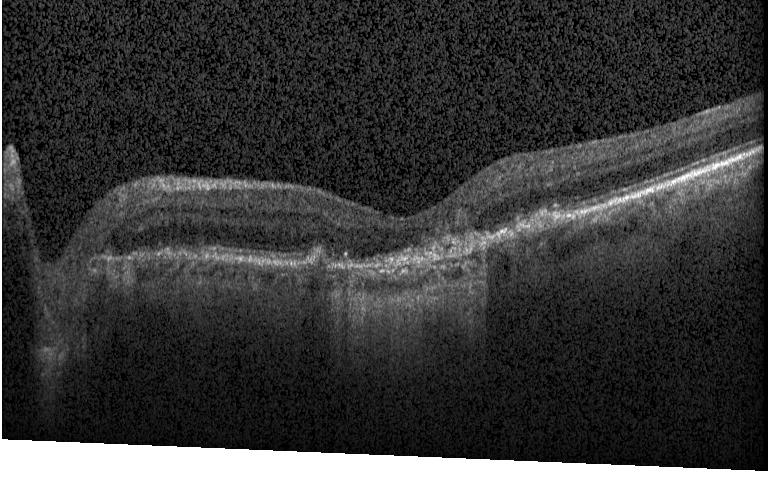

OCT finding: a choroidal neovascular membrane.